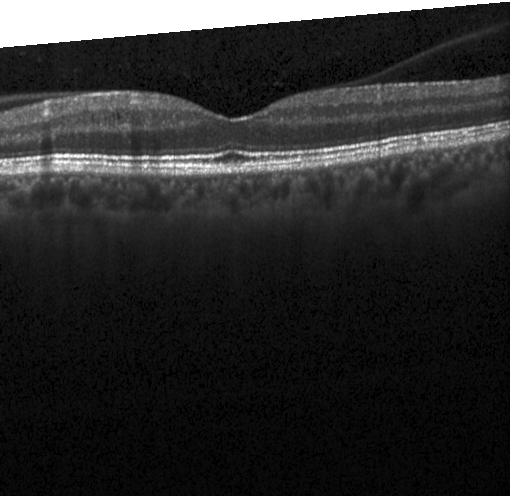 Macular scan; spectral-domain optical coherence tomography; OCT line scan; Heidelberg Spectralis.
This B-scan demonstrates no CNV, DME, or drusen.